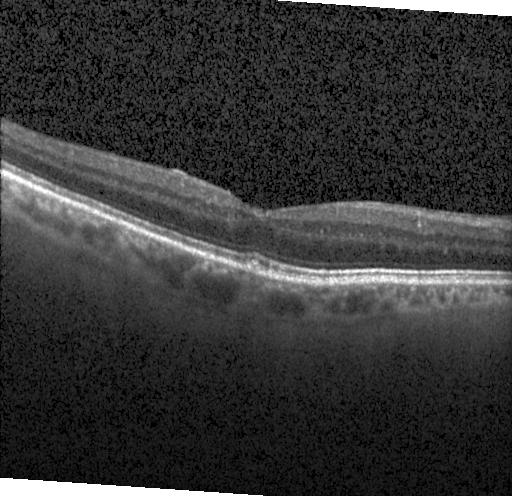

OCT line scan — No choroidal neovascularization, diabetic macular edema, or drusen.